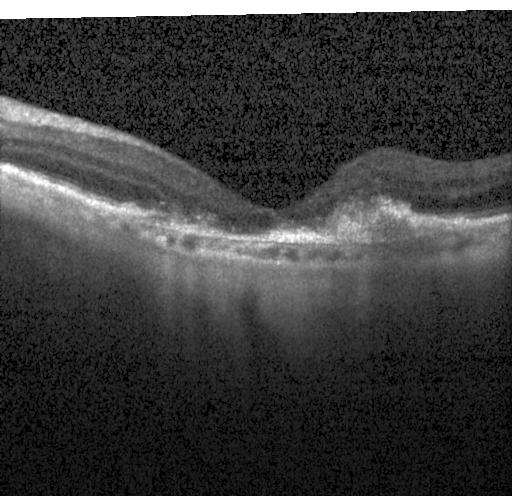 Heidelberg Spectralis OCT system · macular scan · SD-OCT · retinal OCT cross-section. A choroidal neovascular membrane.